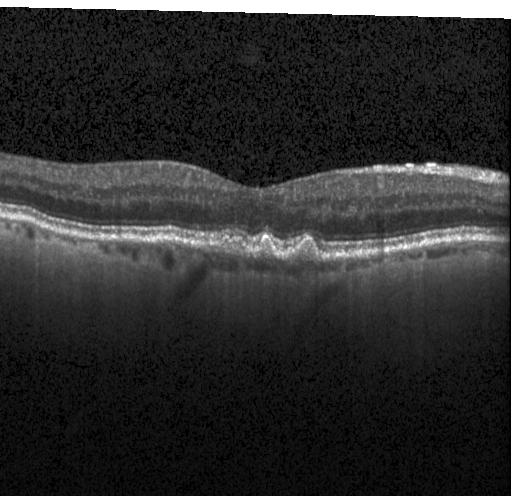
Optical coherence tomography scan — Finding: drusen.